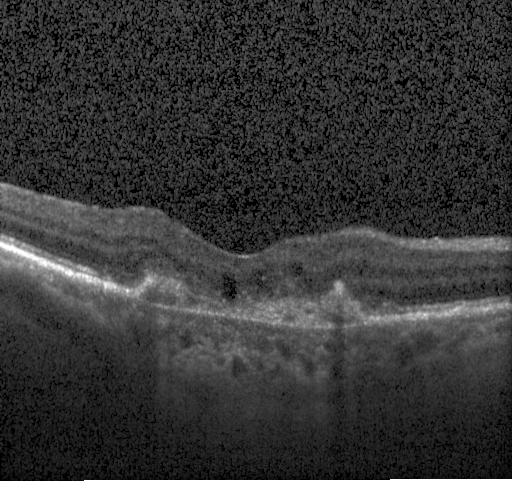
Spectral-domain optical coherence tomography; optical coherence tomography scan. CNV.